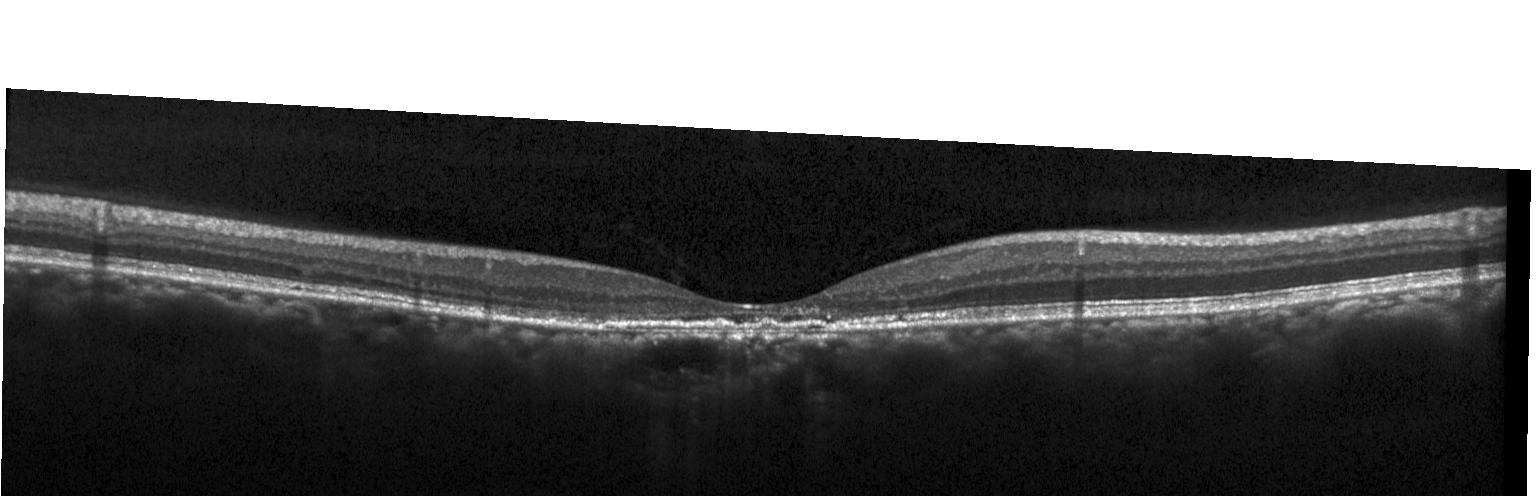 OCT B-scan showing choroidal neovascularization (CNV).